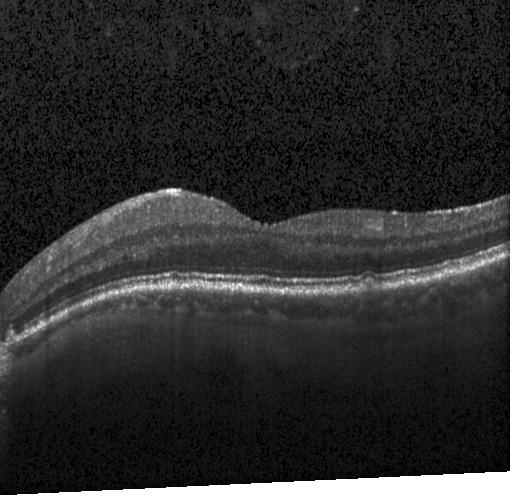 Heidelberg Spectralis OCT system. Retinal OCT cross-section. Macular scan — This B-scan demonstrates drusen.